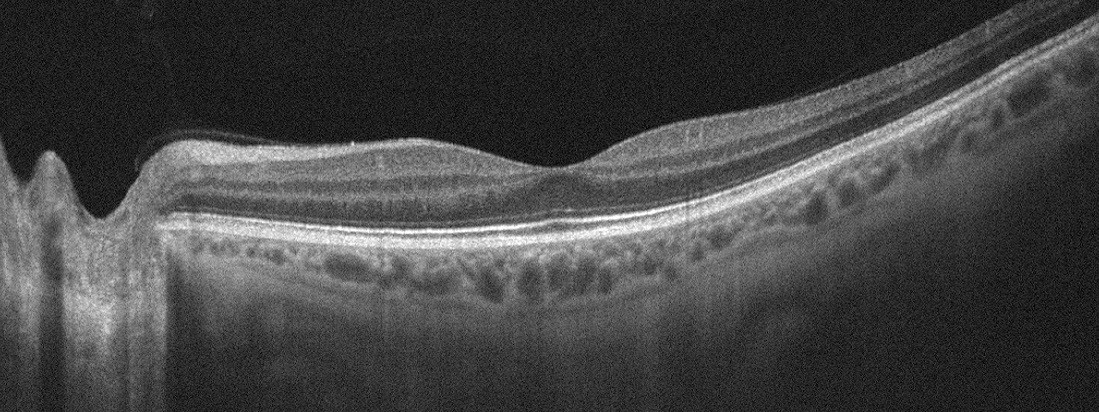 Retinal OCT B-scan; instrument: Optovue Avanti RTVue XR.
Diagnosis: no AMD, DME, ERM, RAO, RVO, or VID.